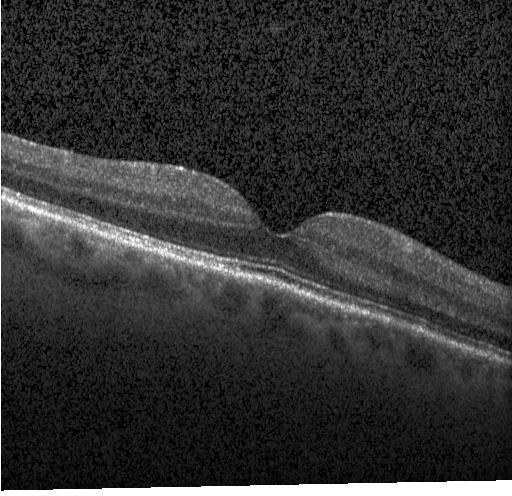 Assessment: no choroidal neovascularization, no diabetic macular edema, and no drusen.